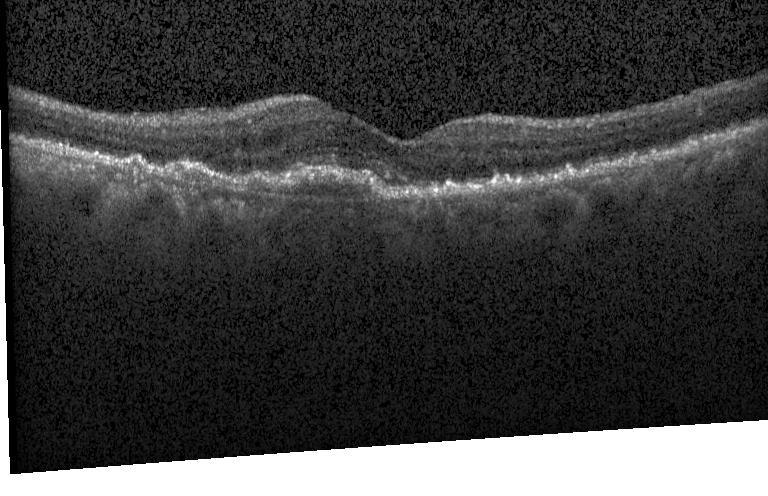
SD-OCT. Optical coherence tomography scan — Impression: a choroidal neovascular membrane.